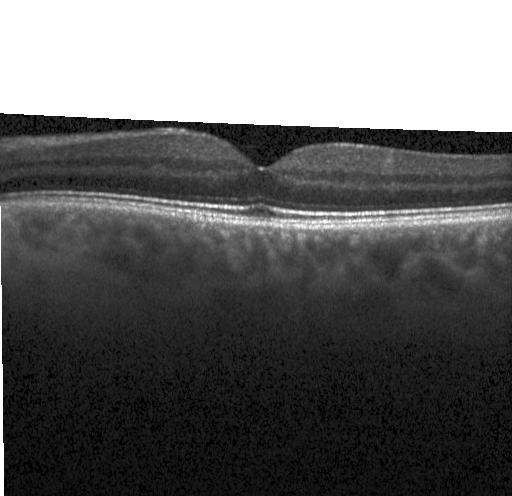
Macular OCT: no choroidal neovascularization, diabetic macular edema, or drusen.